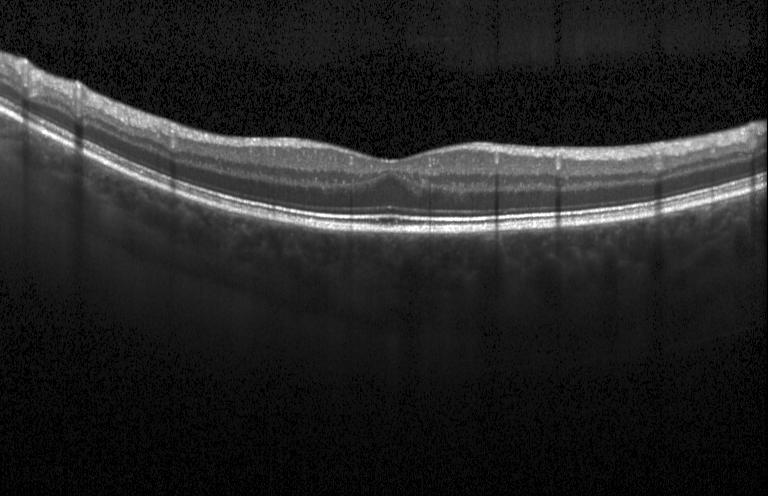

SD-OCT, Heidelberg Spectralis, OCT B-scan — No choroidal neovascularization, diabetic macular edema, or drusen.